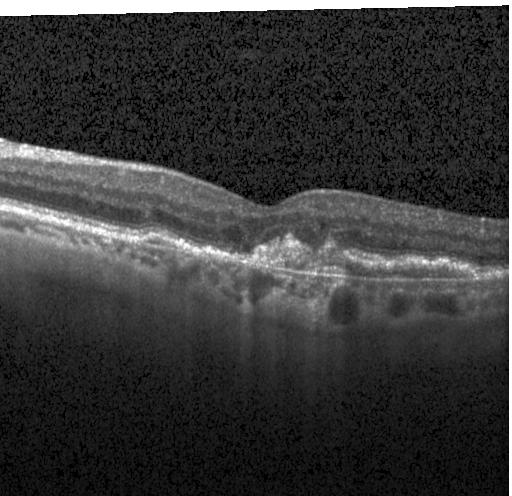

Spectral-domain OCT, OCT B-scan, through the macula. Finding: choroidal neovascularization.